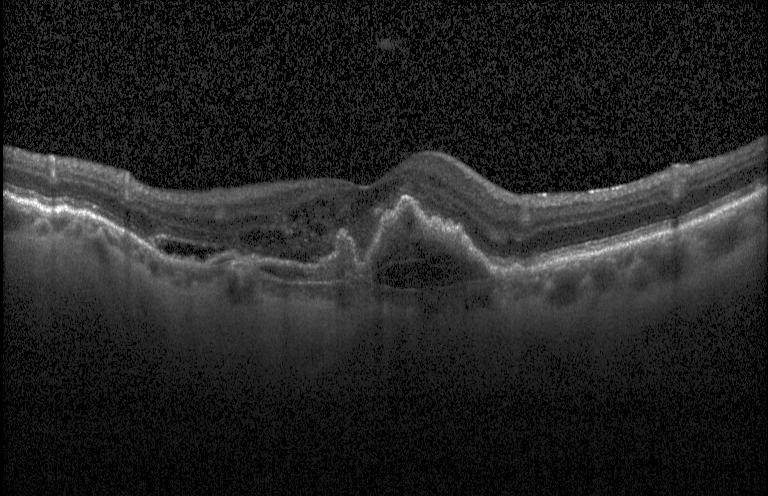 Finding: CNV.